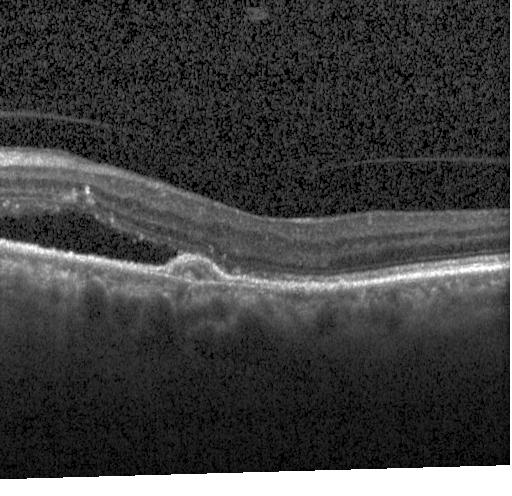

Acquired on a Heidelberg Spectralis, optical coherence tomography scan.
Finding: choroidal neovascularization.